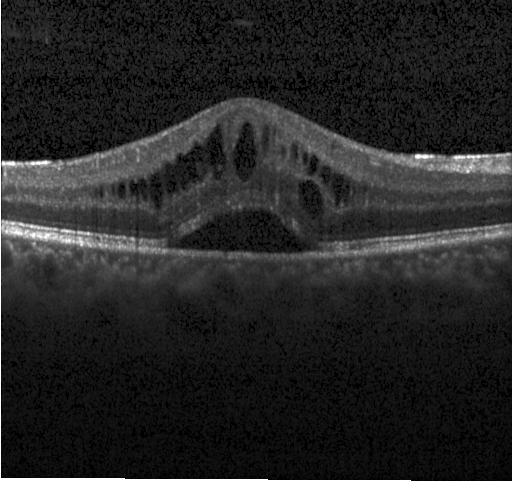
Diagnosis: diabetic macular edema.